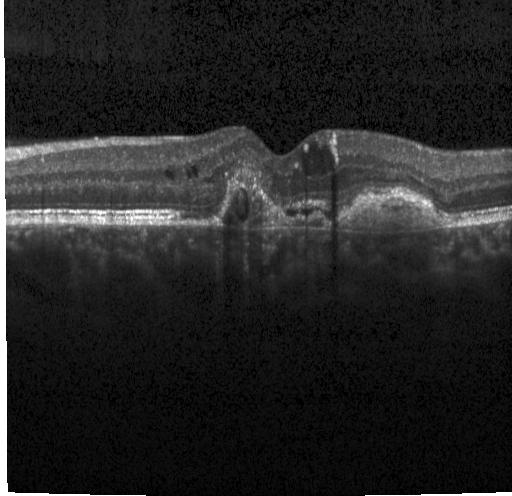
Heidelberg Spectralis OCT system, optical coherence tomography scan, horizontal scan through the fovea. Impression: choroidal neovascularization (CNV).